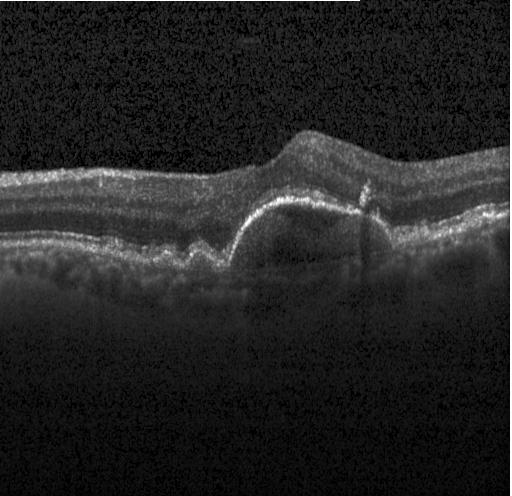
Retinal OCT cross-section · SD-OCT · centered on the fovea · Heidelberg Spectralis OCT system
Dx: multiple drusen.